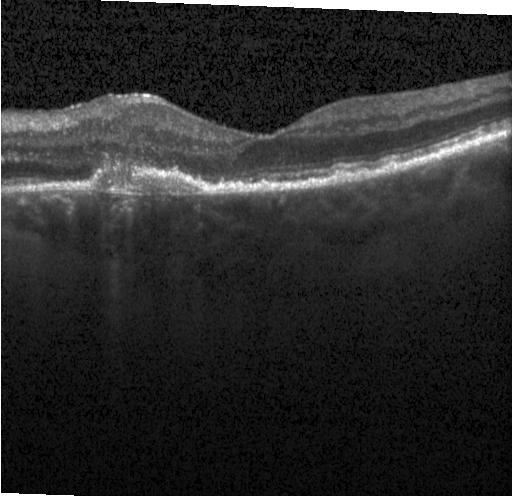
Optical coherence tomography scan
Dx: CNV.